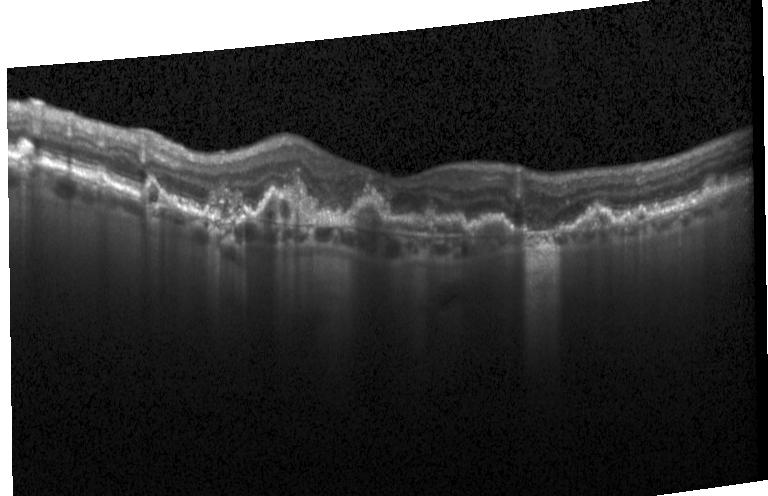

Optical coherence tomography B-scan — Finding: choroidal neovascularization (CNV).